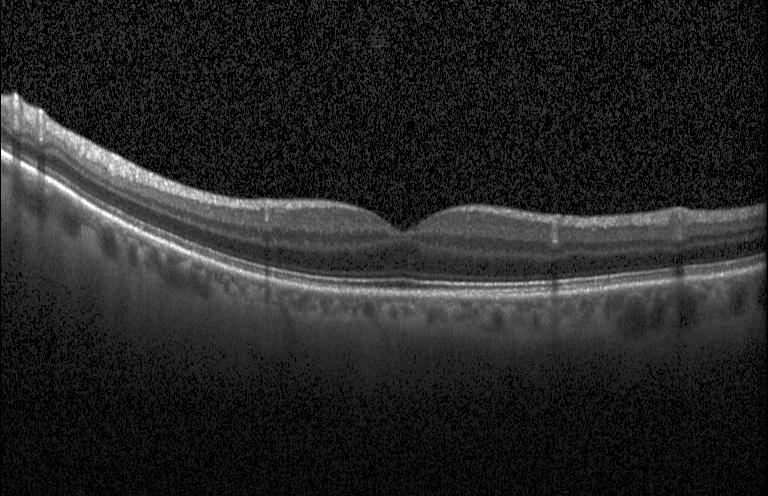 Macular scan. OCT line scan. Spectral-domain optical coherence tomography. Heidelberg Spectralis OCT system.
Macular OCT: no CNV, no DME, and no drusen.